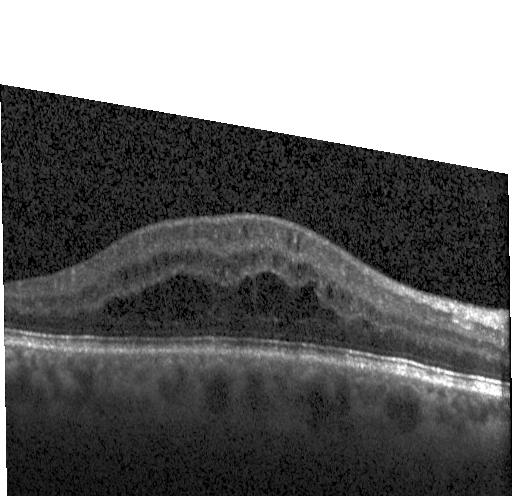

Retinal OCT B-scan · Heidelberg Spectralis OCT system. Finding: diabetic macular edema.